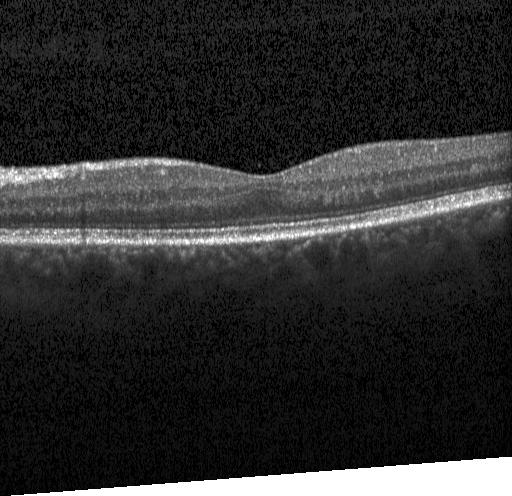 Retinal OCT cross-section showing no CNV, DME, or drusen.